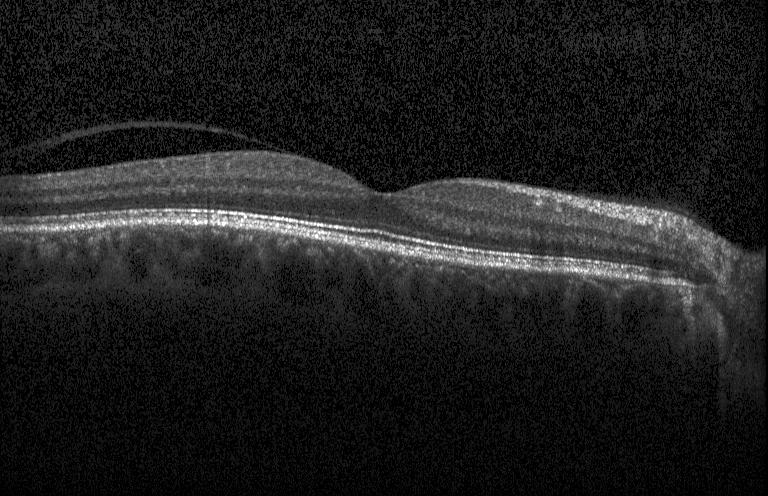
Optical coherence tomography scan, Heidelberg Spectralis, spectral-domain OCT. Finding: no choroidal neovascularization, diabetic macular edema, or drusen.